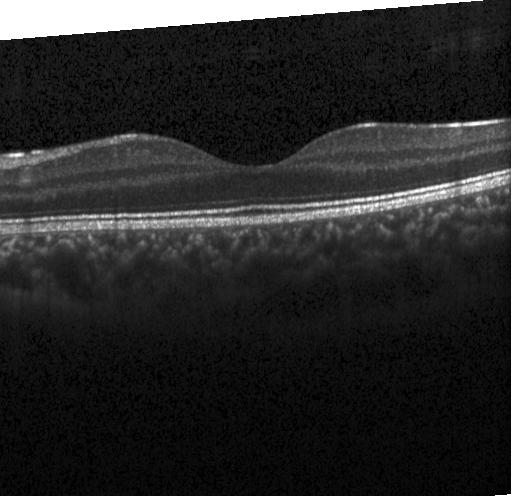
Macular OCT demonstrating no evidence of choroidal neovascularization, diabetic macular edema, or drusen.